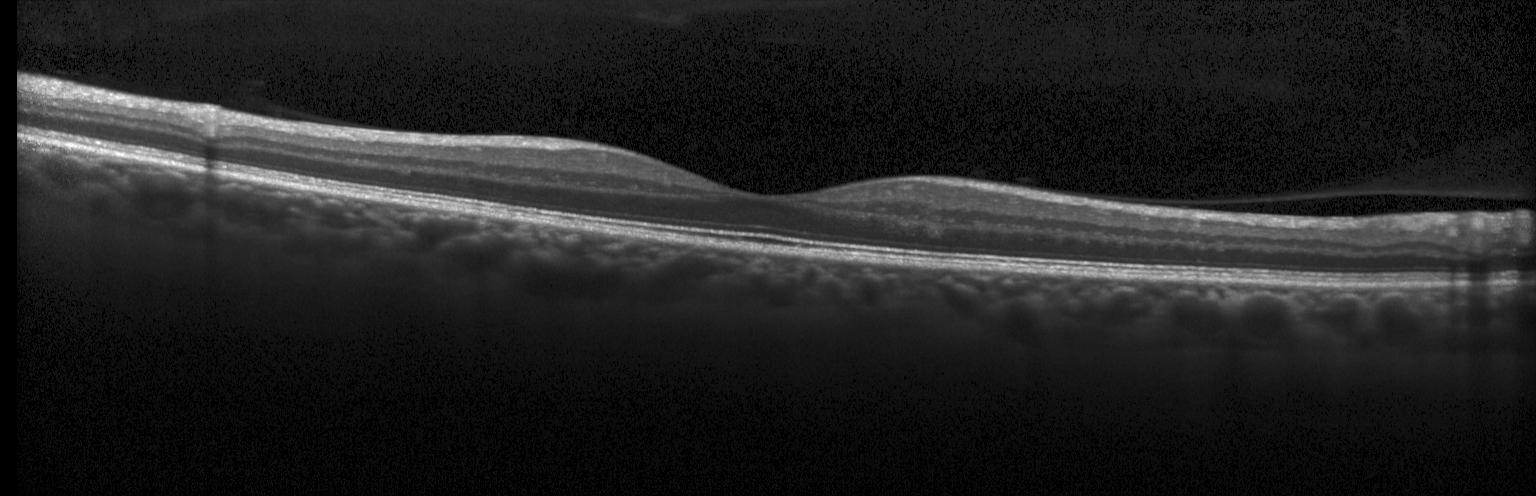

Instrument: Heidelberg Spectralis · OCT line scan · spectral-domain OCT.
The scan shows no CNV, DME, or drusen.